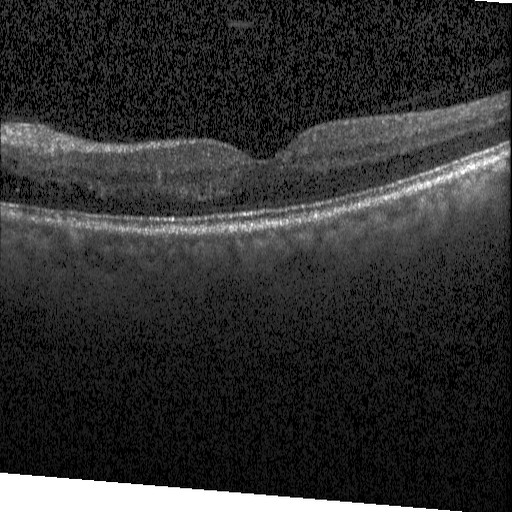 Retinal OCT cross-section showing diabetic macular edema (DME).